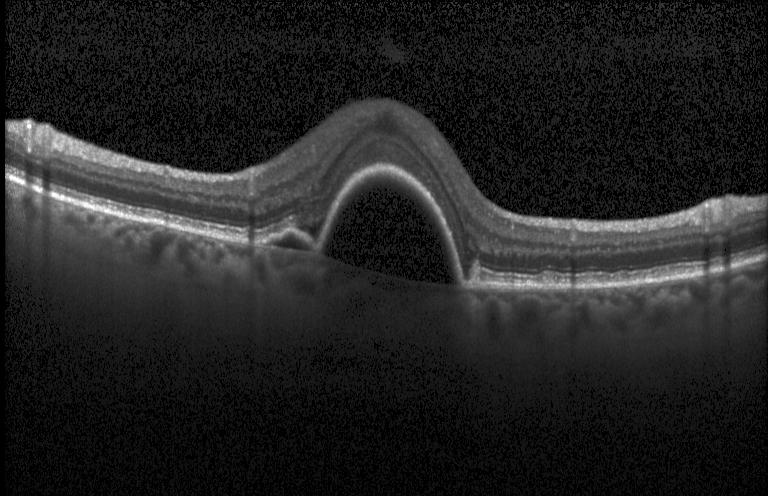 Optical coherence tomography scan. Macular scan — Impression: a choroidal neovascular membrane.